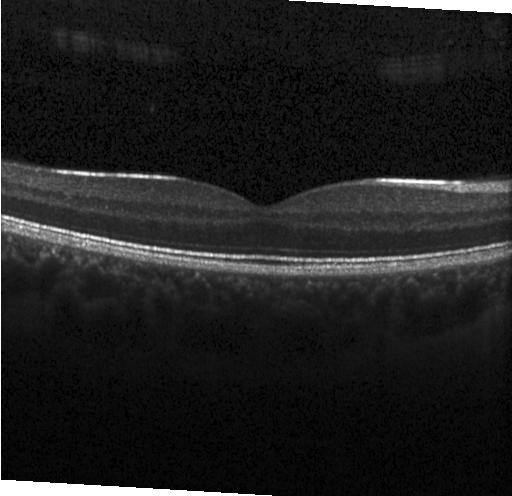
OCT line scan. Spectral-domain optical coherence tomography — Assessment: no choroidal neovascularization, no diabetic macular edema, and no drusen.